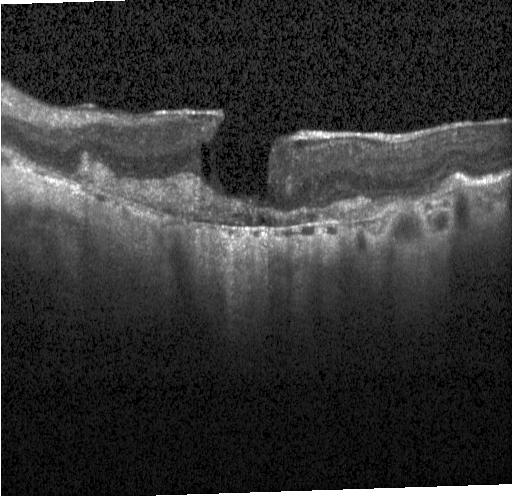

The scan shows choroidal neovascularization (CNV).